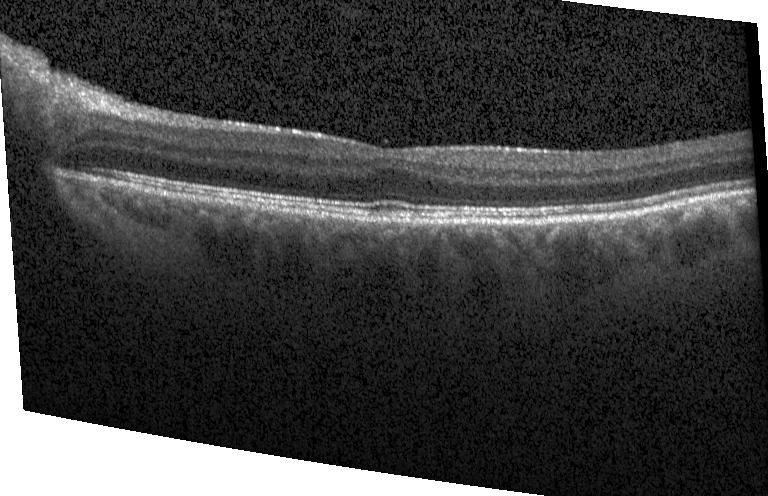
Macular scan · retinal OCT cross-section · Heidelberg Spectralis OCT system · spectral-domain optical coherence tomography. Impression: neither CNV, DME, nor drusen.